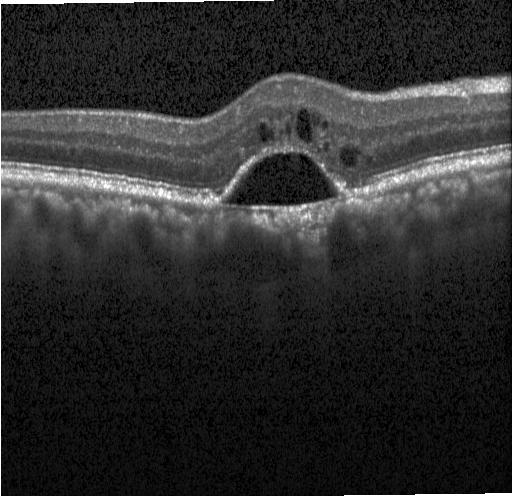
Macular OCT: a choroidal neovascular membrane.